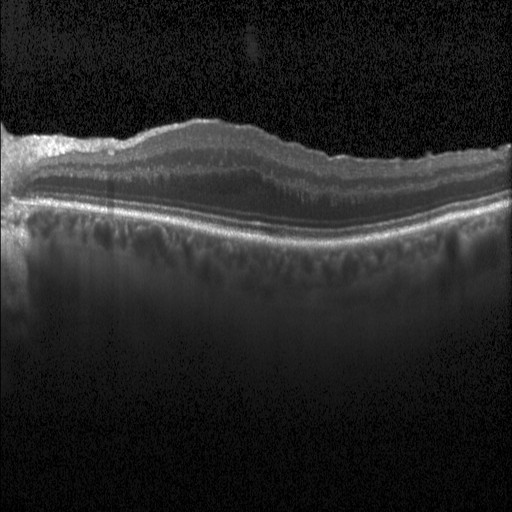 OCT B-scan, fovea-centered.
Macular OCT: DME.